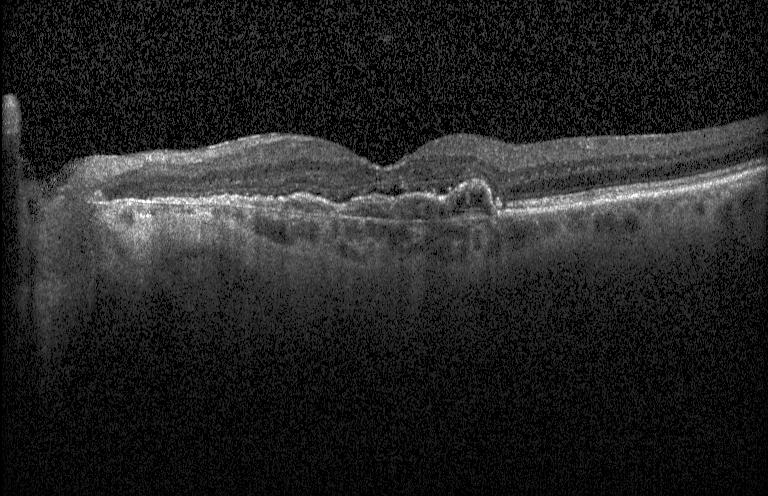
The scan shows CNV.